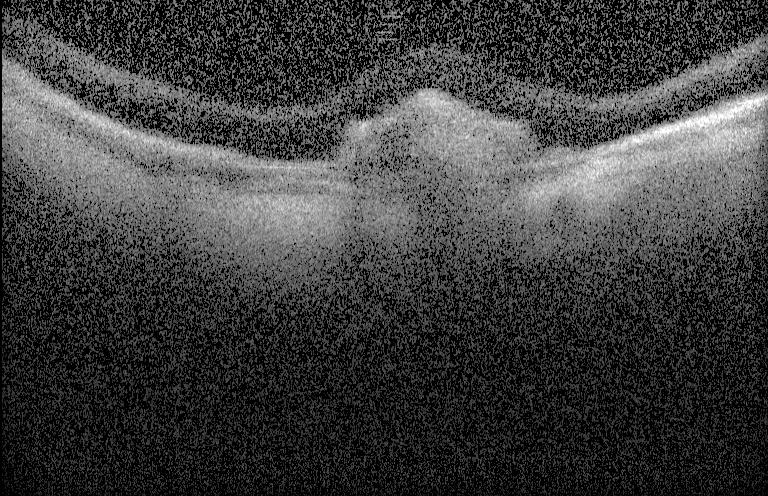
Heidelberg Spectralis, optical coherence tomography B-scan, horizontal scan through the fovea
Finding: CNV.